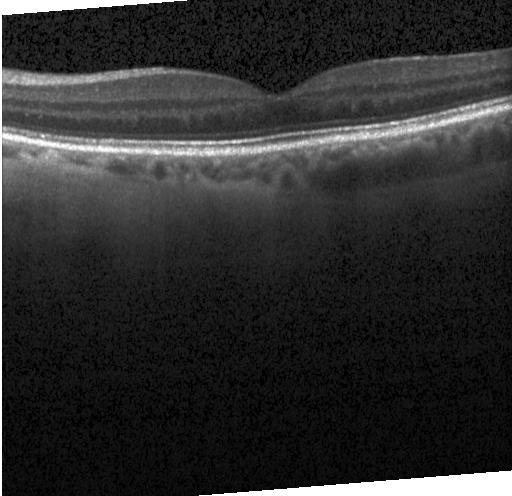 Heidelberg Spectralis OCT system; macular scan; OCT line scan; SD-OCT.
Diagnosis: neither choroidal neovascularization, diabetic macular edema, nor drusen.